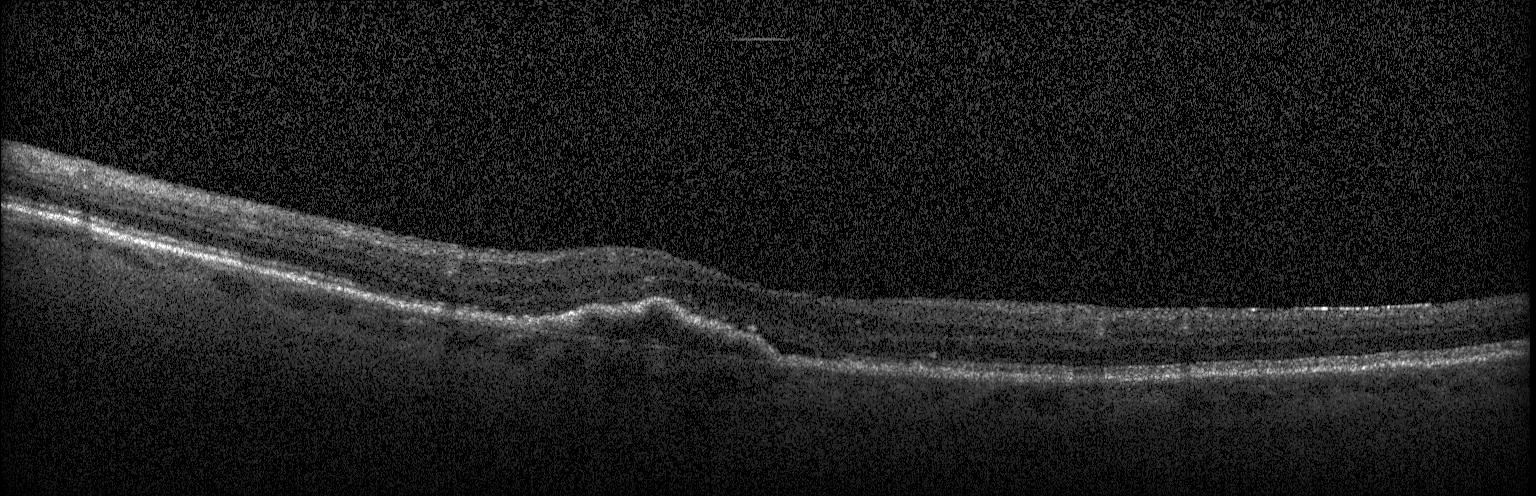
Retinal OCT cross-section showing a choroidal neovascular membrane.